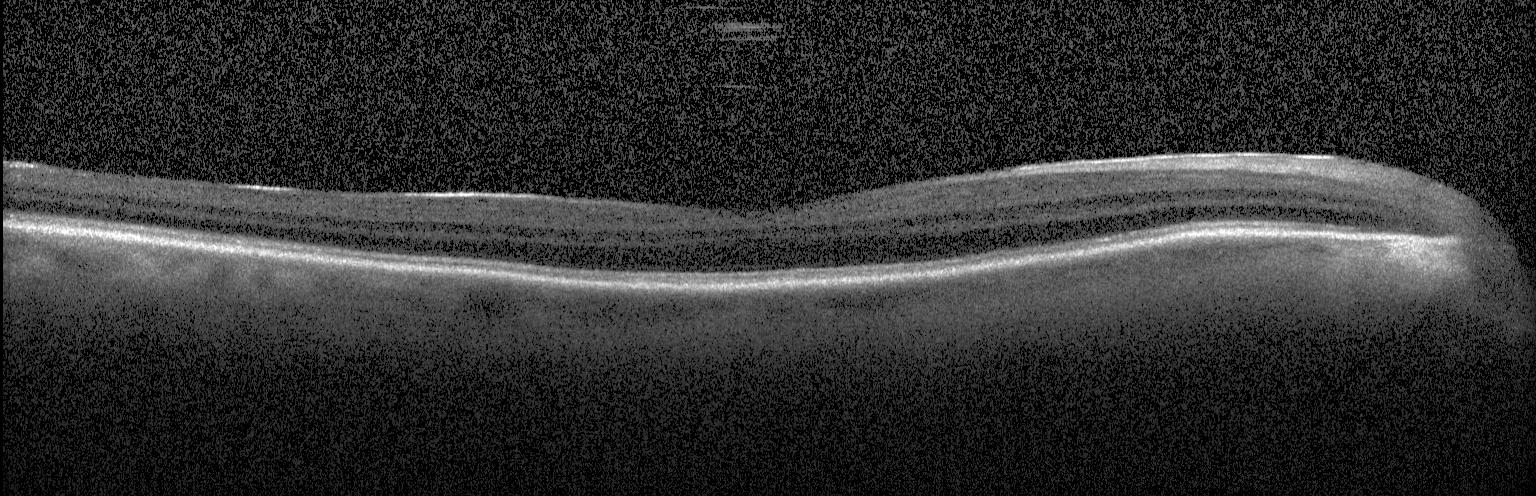

Heidelberg Spectralis · optical coherence tomography B-scan · macular scan — Assessment: no choroidal neovascularization, no diabetic macular edema, and no drusen.